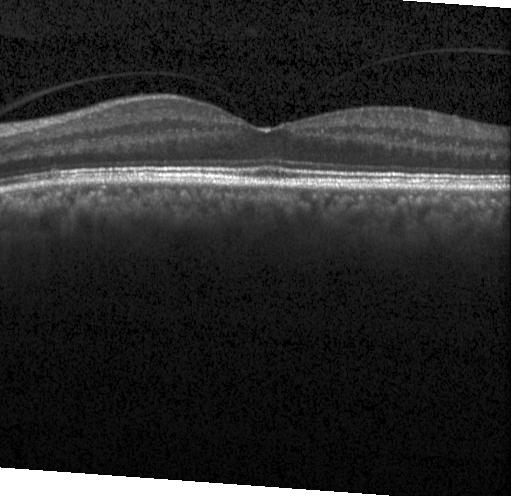

SD-OCT · OCT line scan · fovea-centered. Diagnosis: neither choroidal neovascularization, diabetic macular edema, nor drusen.